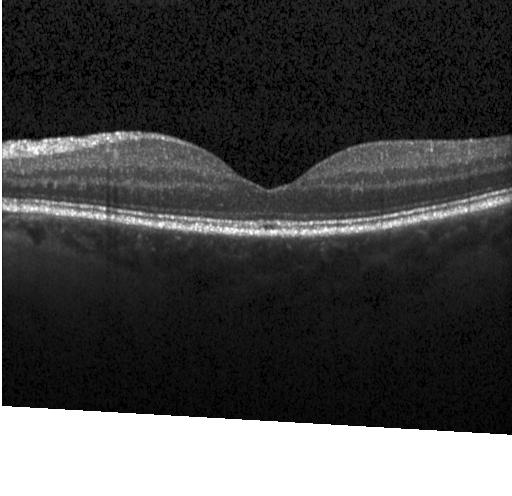
Finding: no evidence of CNV, DME, or drusen.